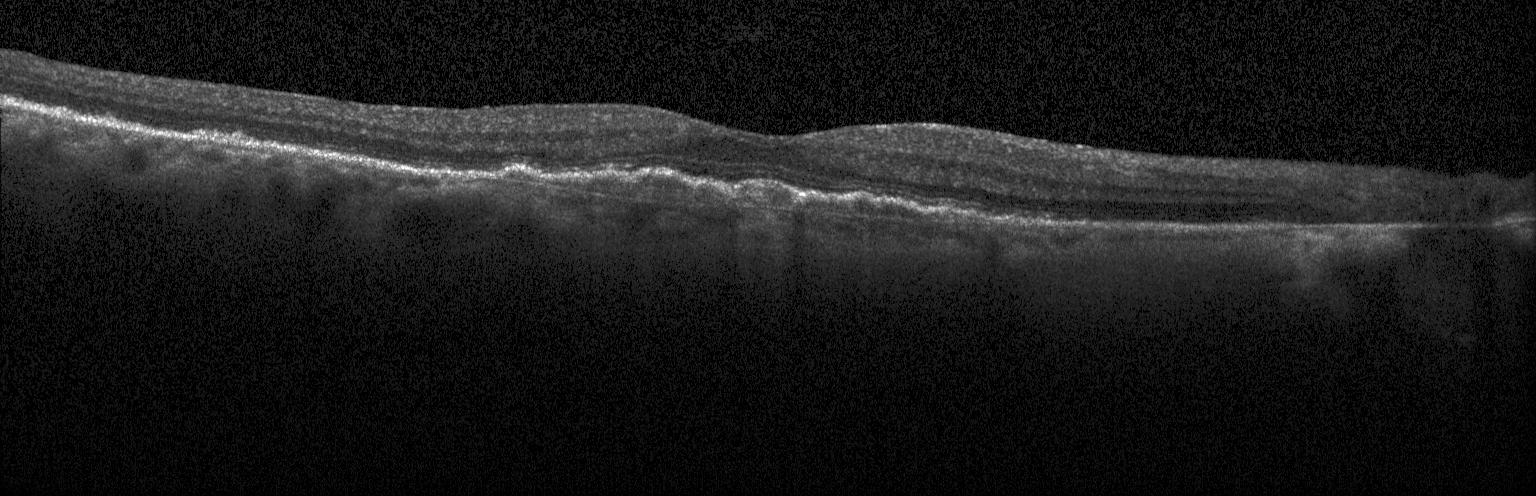
Retinal OCT cross-section — Diagnosis: CNV.